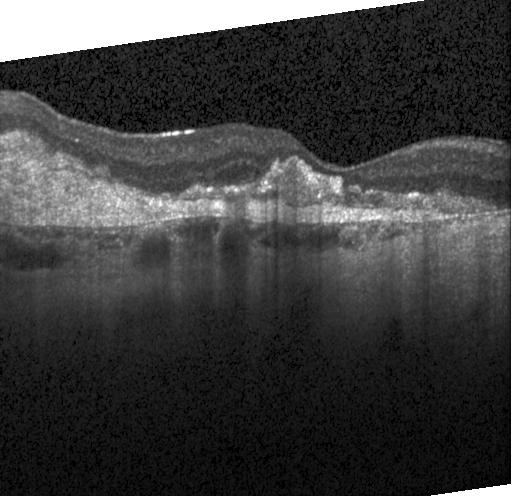
Choroidal neovascularization.